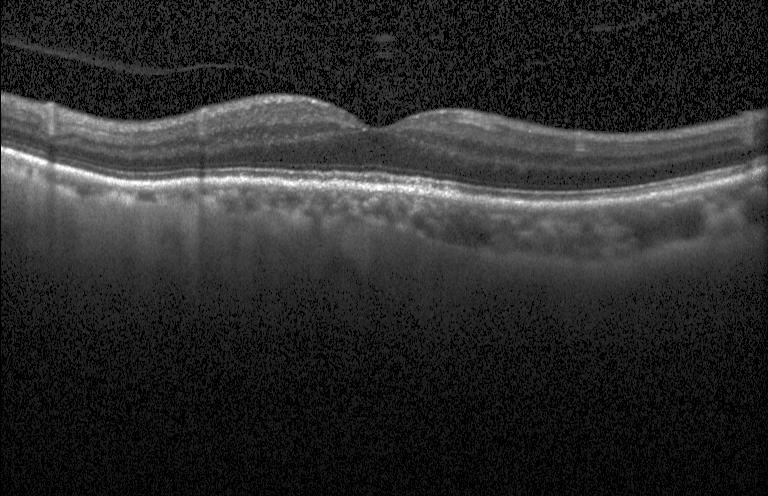
Instrument: Heidelberg Spectralis. SD-OCT. Macular scan. Retinal OCT B-scan. Finding: neither choroidal neovascularization, diabetic macular edema, nor drusen.